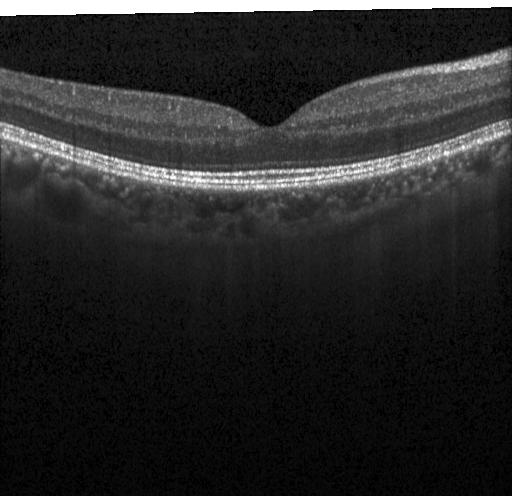

Spectral-domain optical coherence tomography; horizontal scan through the fovea; retinal OCT cross-section.
Assessment: no evidence of choroidal neovascularization, diabetic macular edema, or drusen.